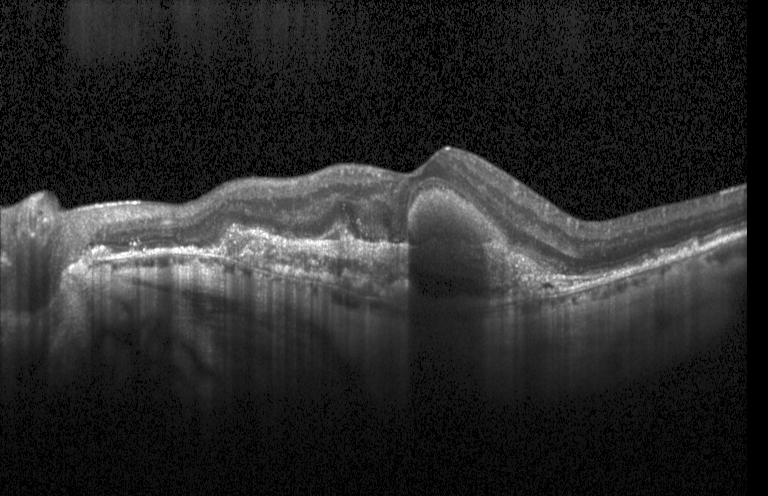
Diagnosis: choroidal neovascularization.